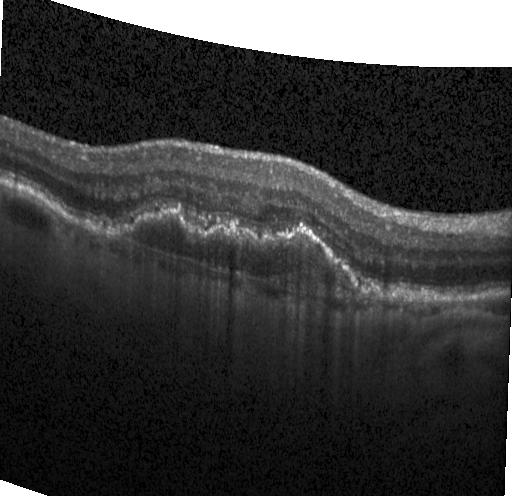 OCT line scan
Choroidal neovascularization.